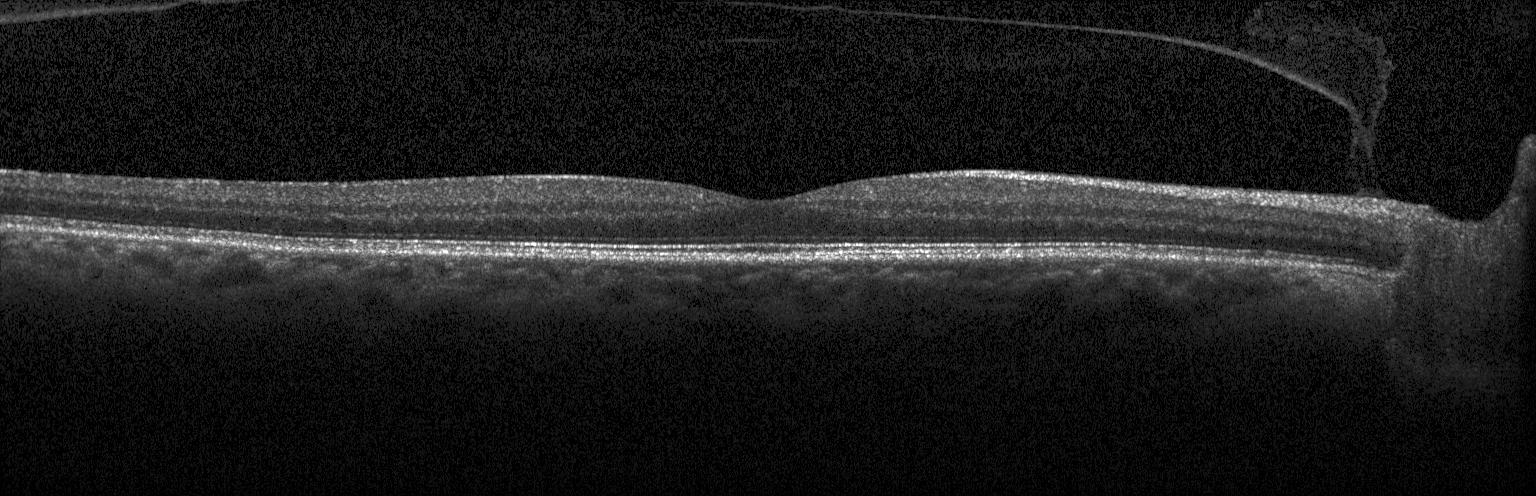
Acquired on a Heidelberg Spectralis · through the macula · SD-OCT · optical coherence tomography B-scan.
Finding: no evidence of choroidal neovascularization, diabetic macular edema, or drusen.